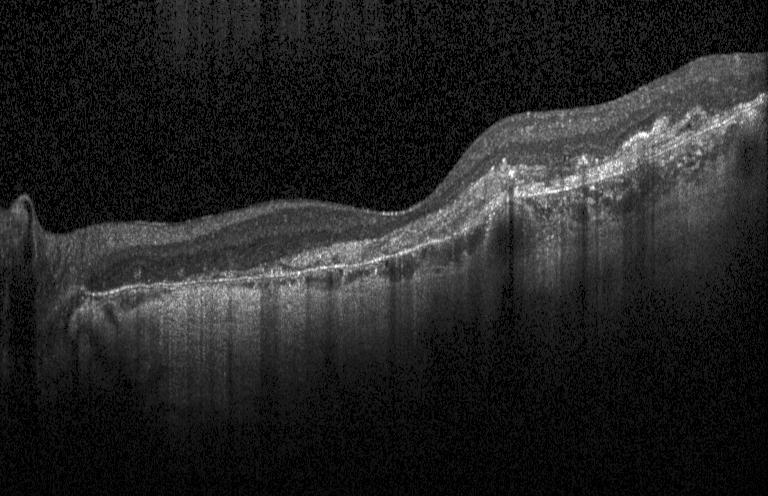

Impression: a choroidal neovascular membrane.